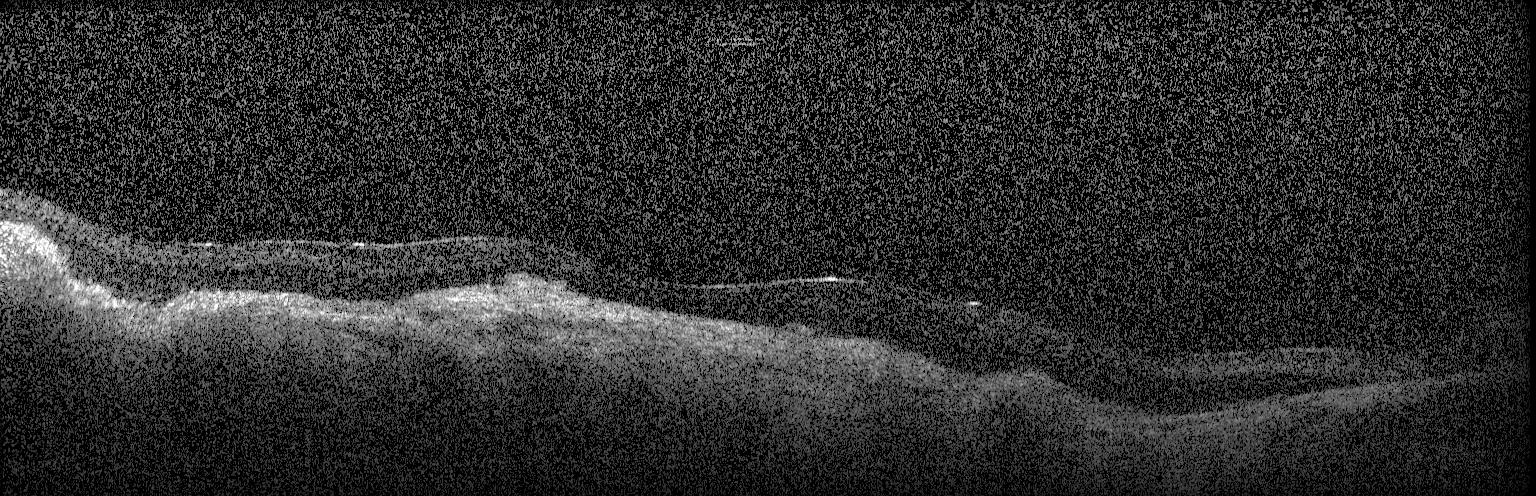 Impression: choroidal neovascularization.